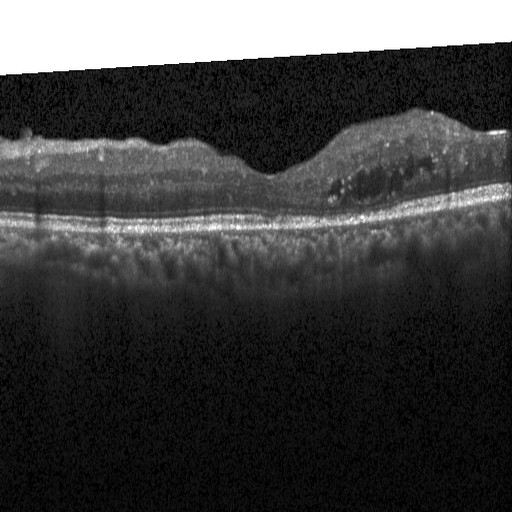
Horizontal scan through the fovea, retinal OCT cross-section, Heidelberg Spectralis.
Diabetic macular edema (DME).